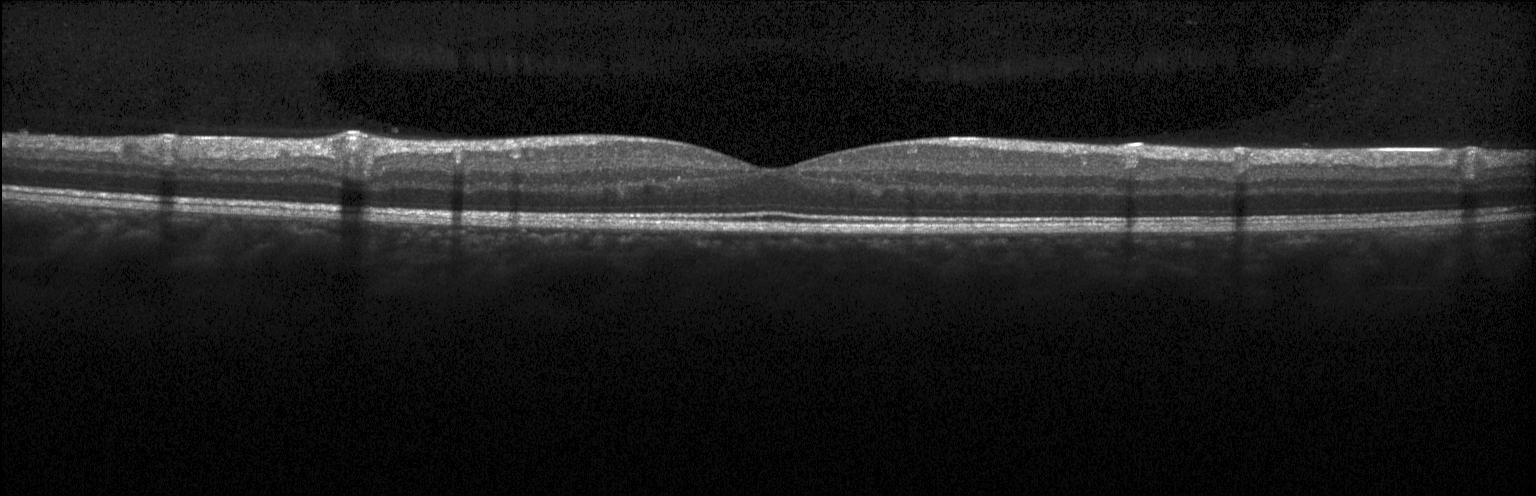

Through the macula. Optical coherence tomography B-scan. Heidelberg Spectralis
Finding: neither choroidal neovascularization, diabetic macular edema, nor drusen.